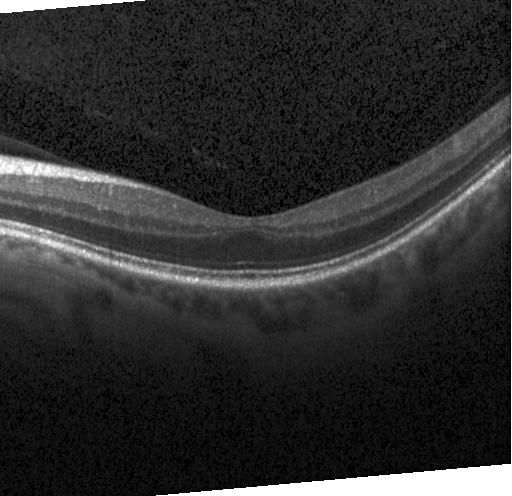 Retinal OCT cross-section
Finding: no choroidal neovascularization, no diabetic macular edema, and no drusen.